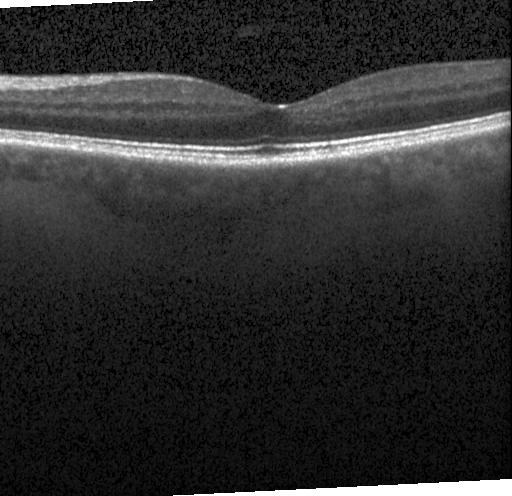
Optical coherence tomography B-scan
Diagnosis: no CNV, no DME, and no drusen.